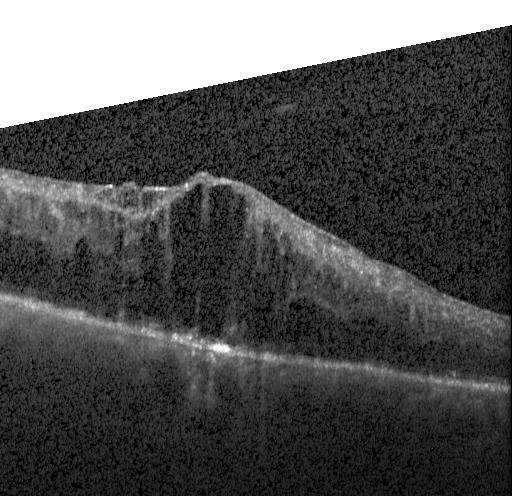

Finding: diabetic macular edema.